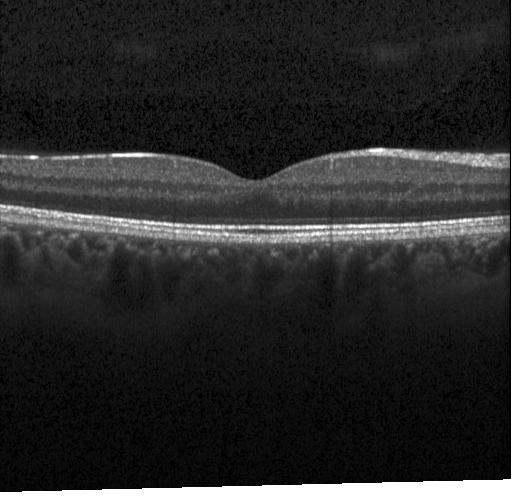

Macular scan; Heidelberg Spectralis OCT system; OCT line scan; spectral-domain optical coherence tomography — OCT finding: neither choroidal neovascularization, diabetic macular edema, nor drusen.